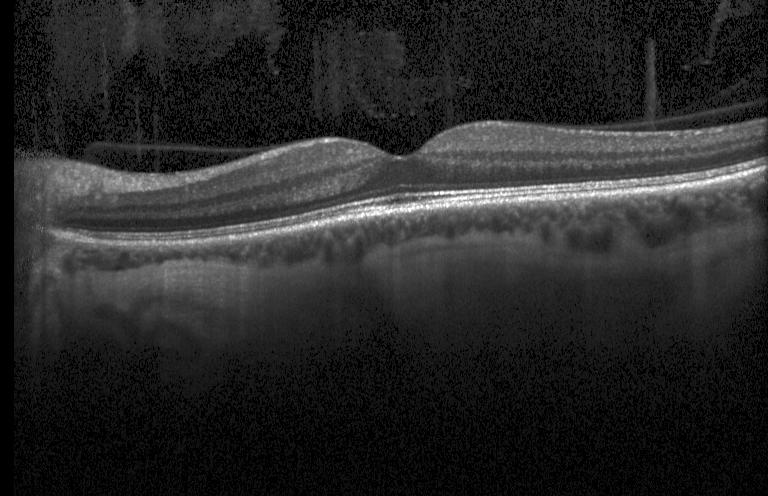 OCT scan showing neither choroidal neovascularization, diabetic macular edema, nor drusen.